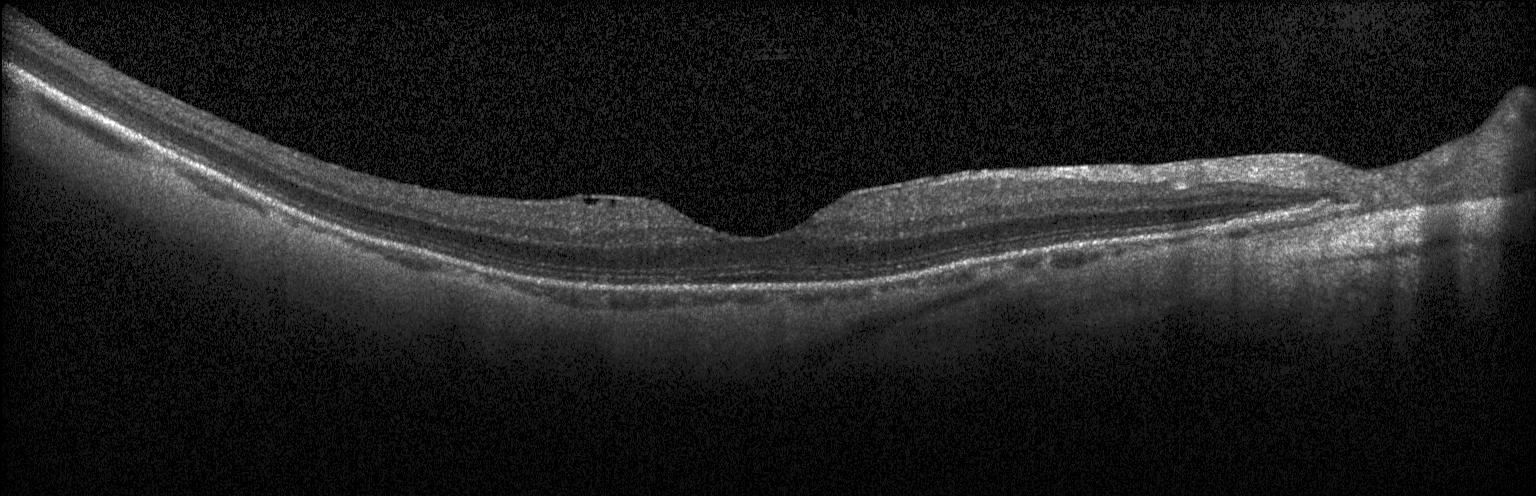

Fovea-centered · OCT B-scan.
Impression: no choroidal neovascularization, no diabetic macular edema, and no drusen.